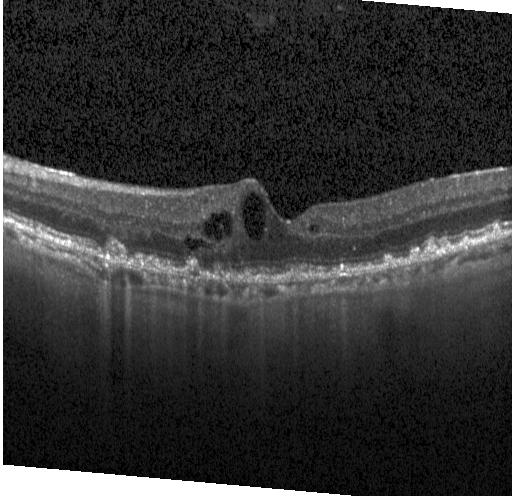

Assessment: a choroidal neovascular membrane.